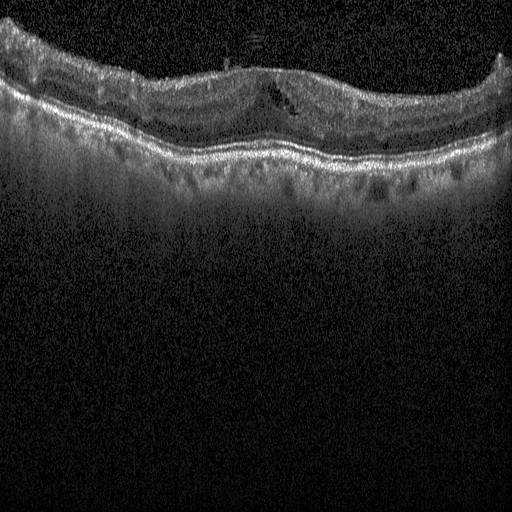 Retinal OCT cross-section.
Assessment: DME.